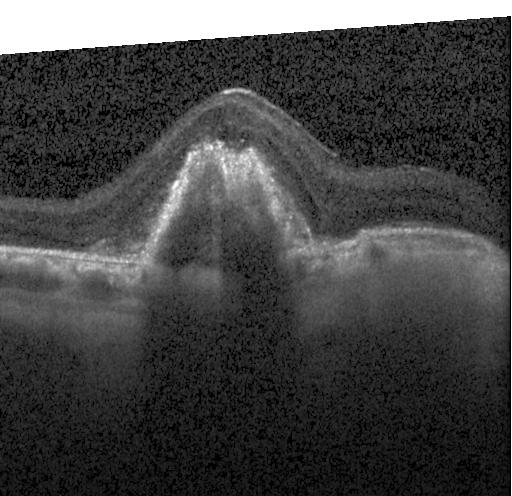
Finding: a choroidal neovascular membrane.